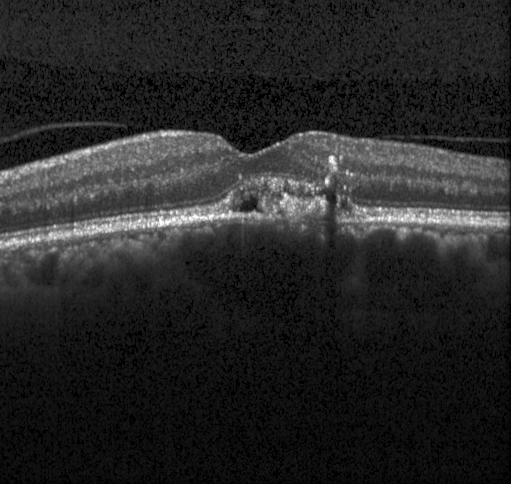

Retinal OCT B-scan, macular scan, Heidelberg Spectralis — Impression: choroidal neovascularization.